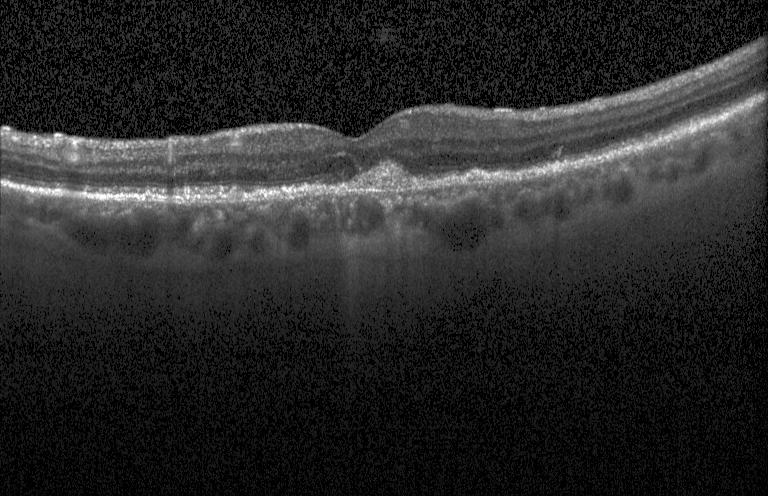
Retinal OCT cross-section. Instrument: Heidelberg Spectralis. Centered on the fovea. Spectral-domain OCT. Diagnosis: a choroidal neovascular membrane.